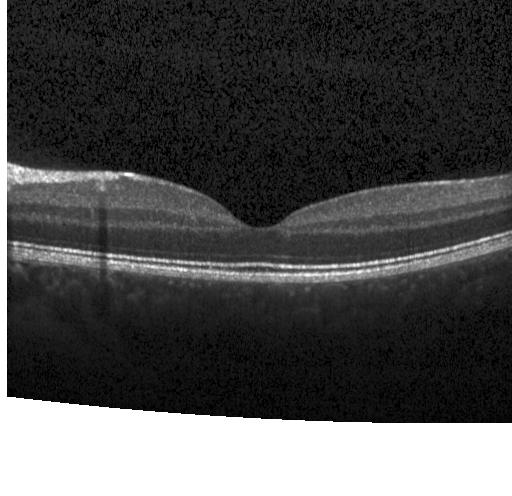

Retinal OCT B-scan; instrument: Heidelberg Spectralis.
This B-scan demonstrates no choroidal neovascularization, no diabetic macular edema, and no drusen.